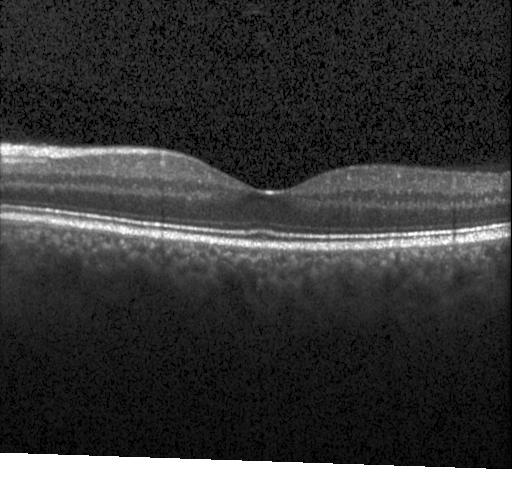 Macular OCT demonstrating no choroidal neovascularization, diabetic macular edema, or drusen.